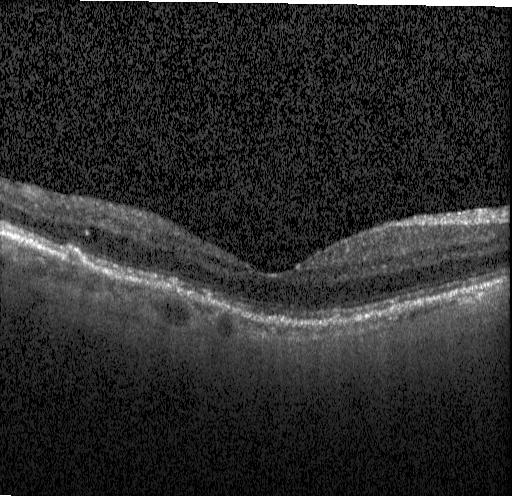

Spectral-domain OCT B-scan: drusen.